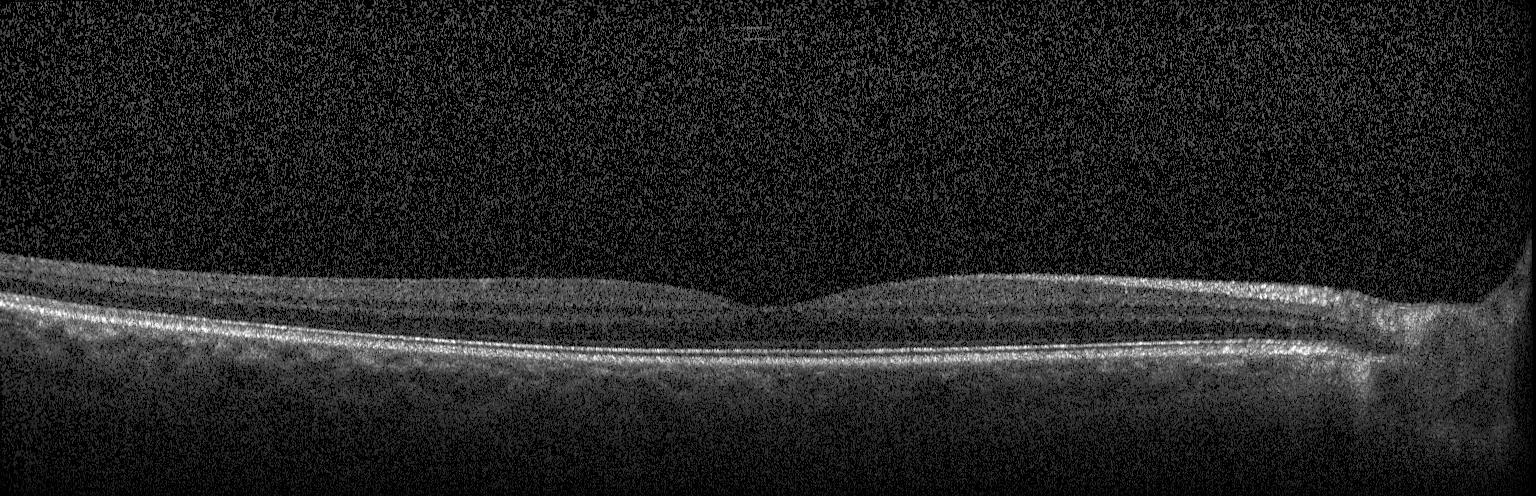
OCT line scan. Heidelberg Spectralis. Horizontal scan through the fovea
Impression: neither CNV, DME, nor drusen.